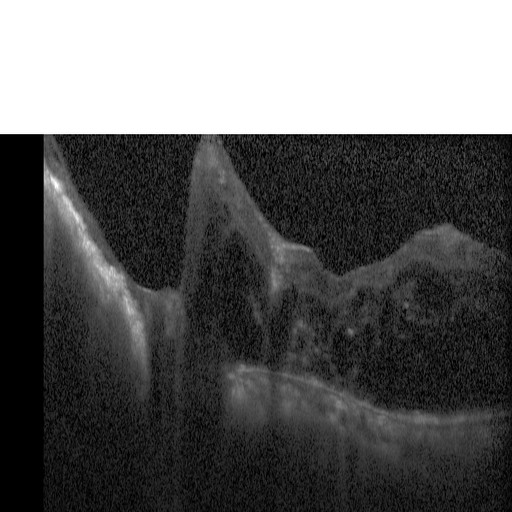

The scan shows diabetic macular edema (DME).